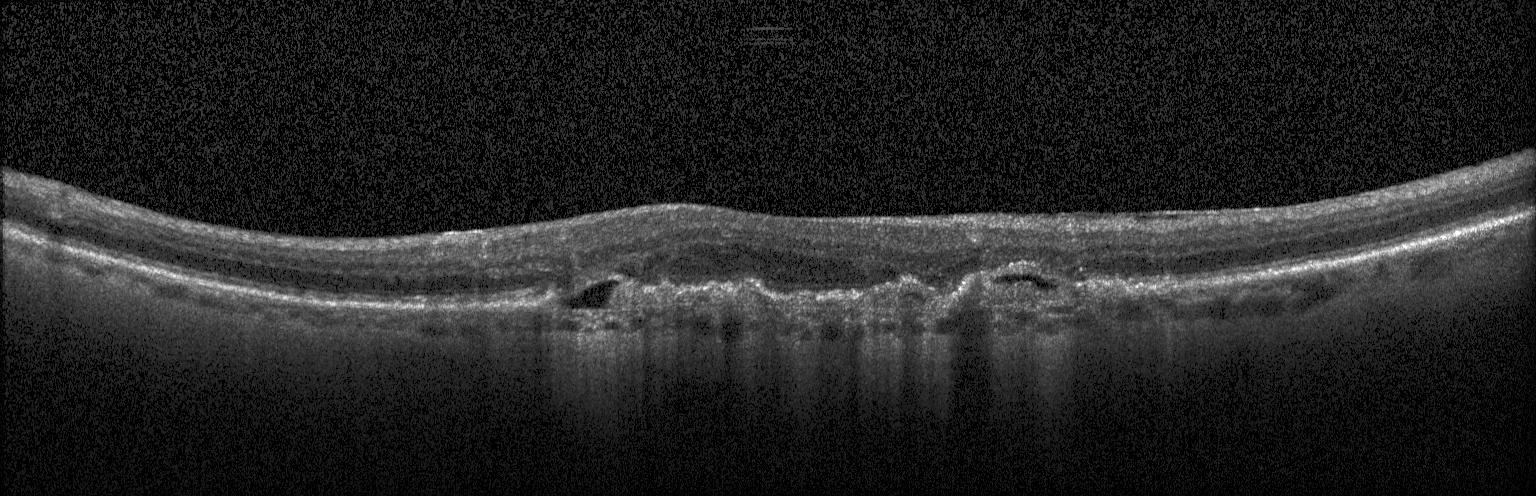 Macular OCT: choroidal neovascularization.